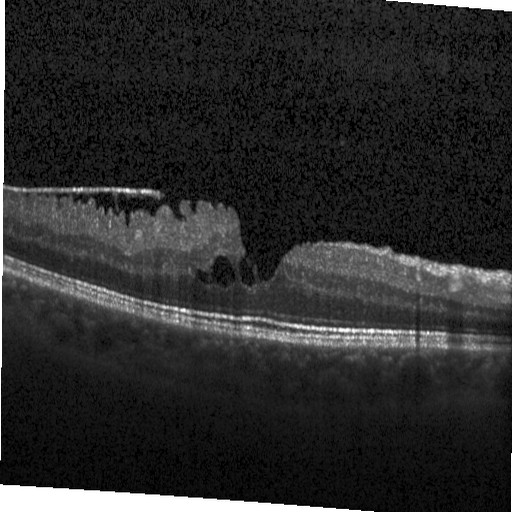

Optical coherence tomography B-scan
This B-scan demonstrates diabetic macular edema.